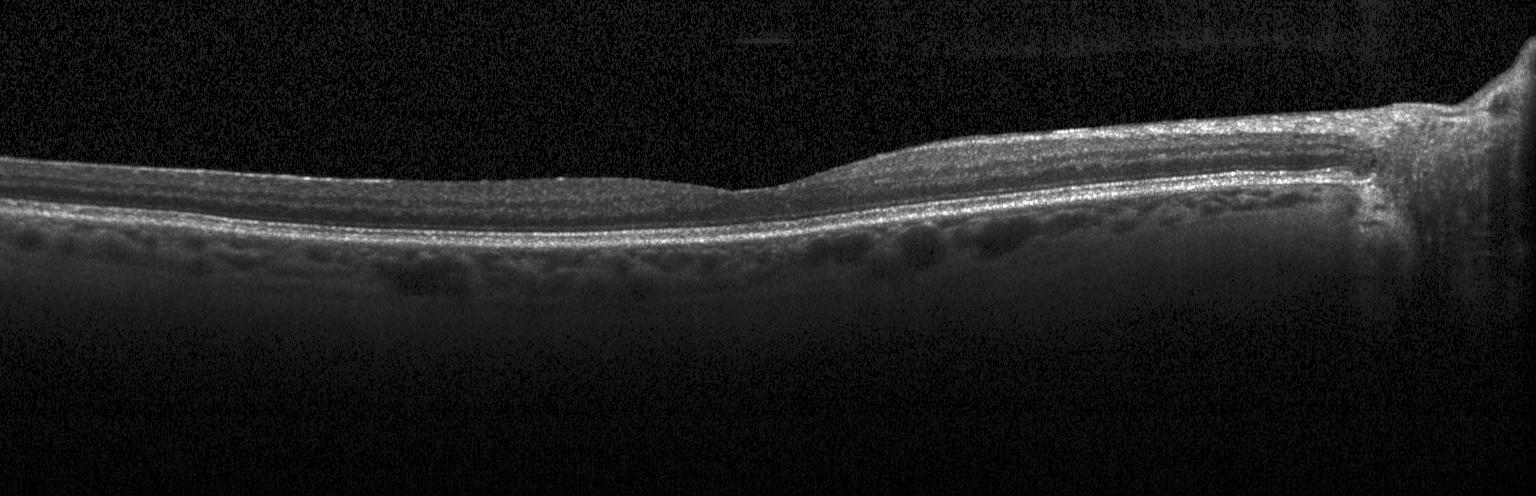

Spectral-domain optical coherence tomography. OCT line scan. OCT finding: no evidence of choroidal neovascularization, diabetic macular edema, or drusen.